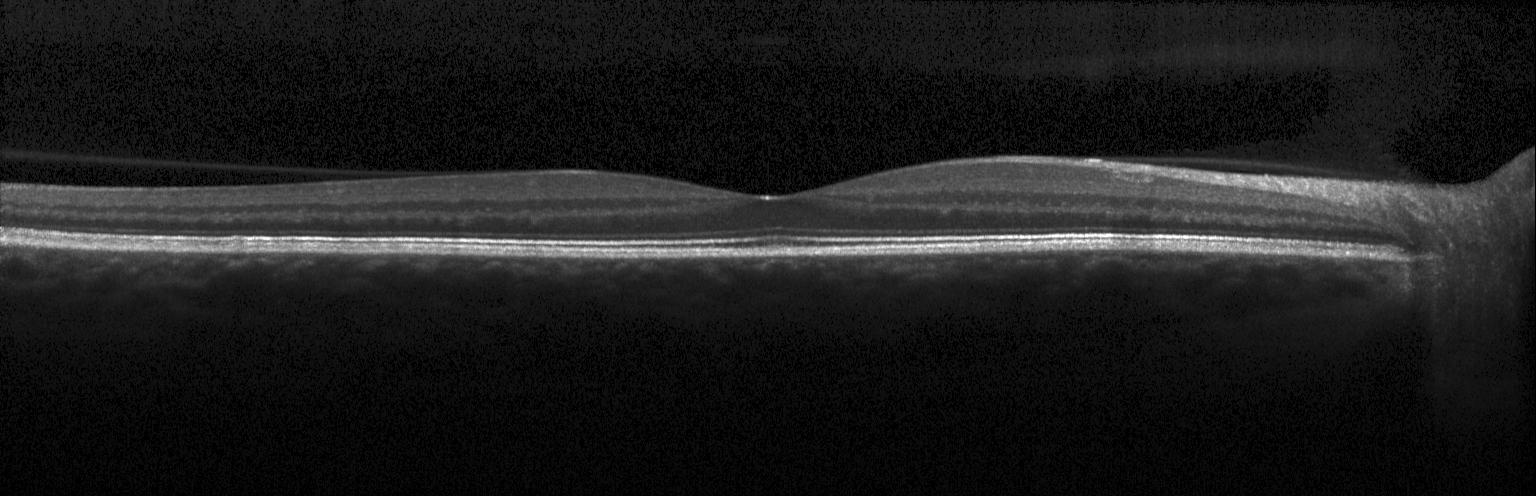

Impression: no choroidal neovascularization, diabetic macular edema, or drusen.